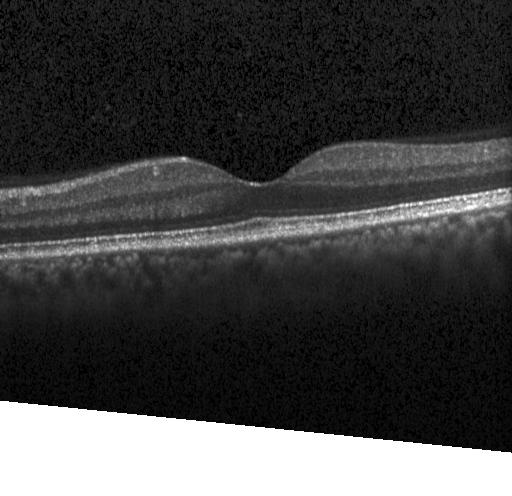

Retinal OCT B-scan — Diagnosis: no choroidal neovascularization, diabetic macular edema, or drusen.